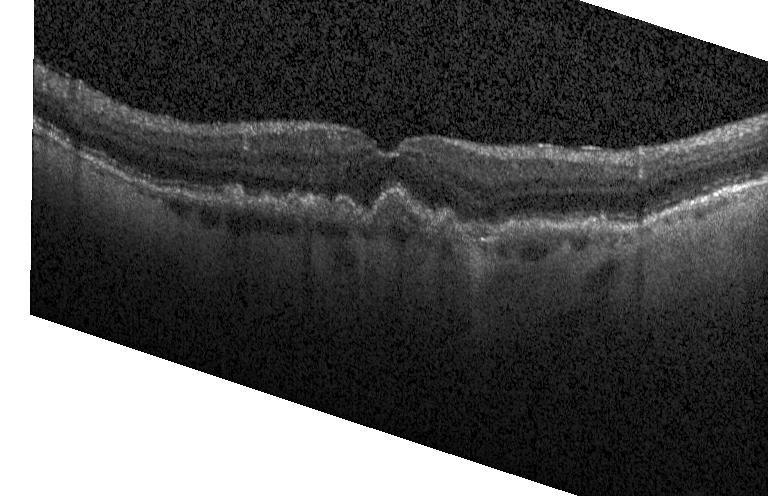

SD-OCT; retinal OCT B-scan
Macular OCT: choroidal neovascularization (CNV).